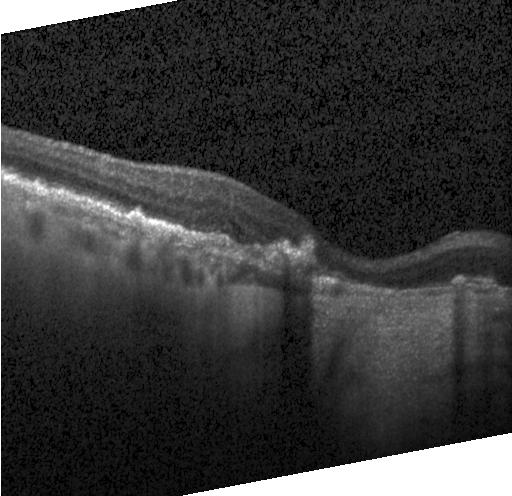
Heidelberg Spectralis, fovea-centered, SD-OCT, optical coherence tomography scan — Finding: CNV.